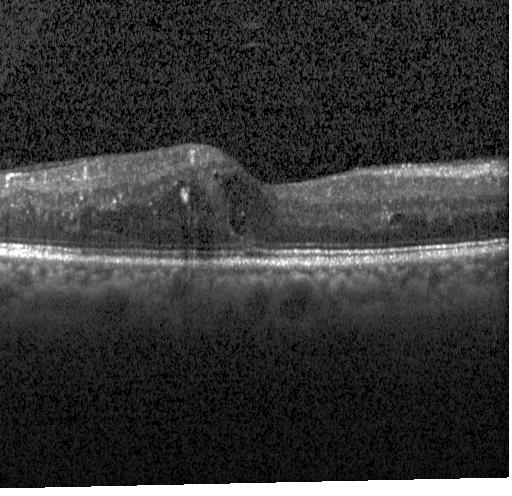

Fovea-centered; spectral-domain optical coherence tomography; optical coherence tomography scan.
Dx: diabetic macular edema (DME).